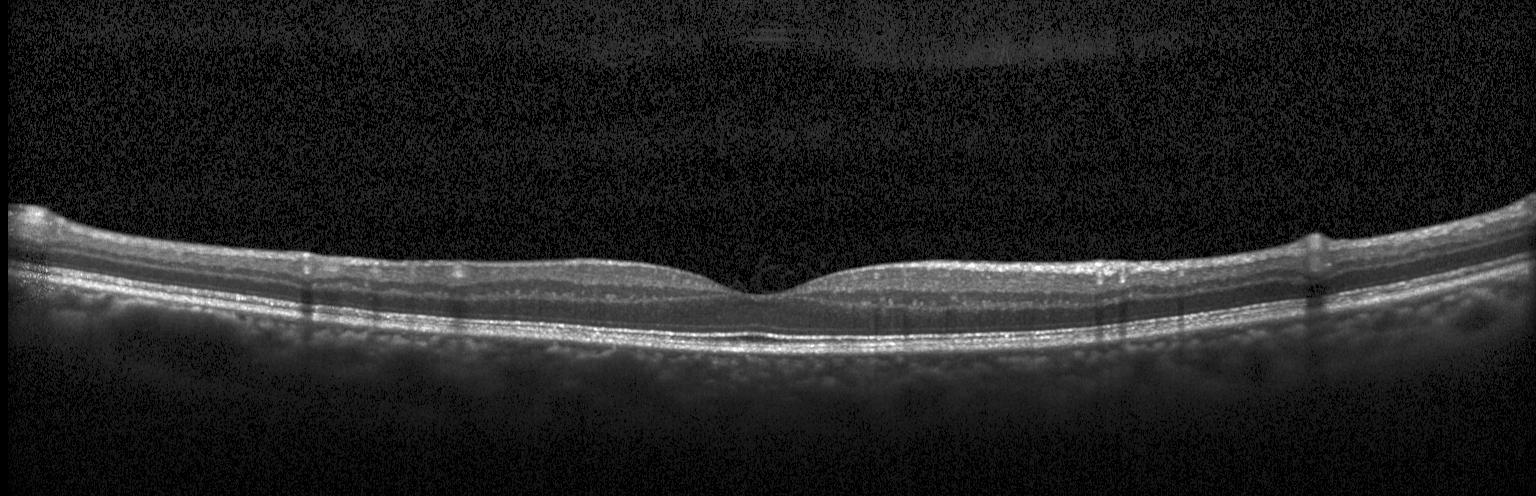
Heidelberg Spectralis OCT system · centered on the fovea · retinal OCT cross-section · spectral-domain optical coherence tomography
The scan shows no choroidal neovascularization, diabetic macular edema, or drusen.